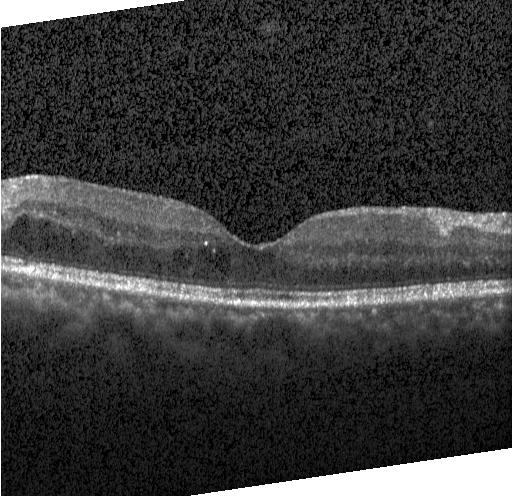
Heidelberg Spectralis; SD-OCT; retinal OCT cross-section.
Finding: diabetic macular edema (DME).